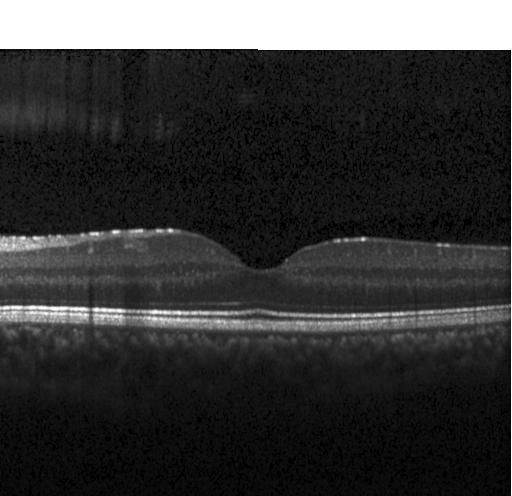

OCT line scan.
Impression: no evidence of choroidal neovascularization, diabetic macular edema, or drusen.